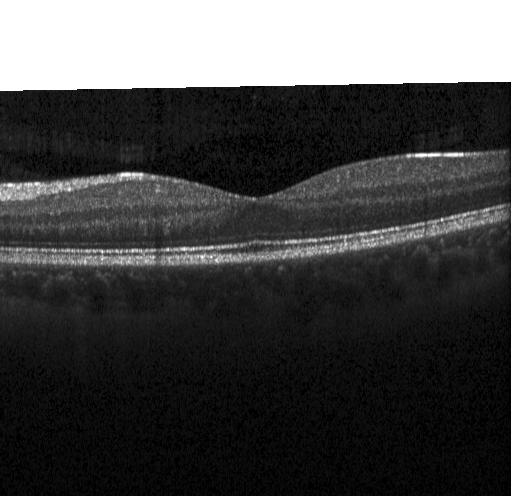
Spectral-domain OCT. Centered on the fovea. Optical coherence tomography scan. Instrument: Heidelberg Spectralis
Macular OCT: no evidence of CNV, DME, or drusen.